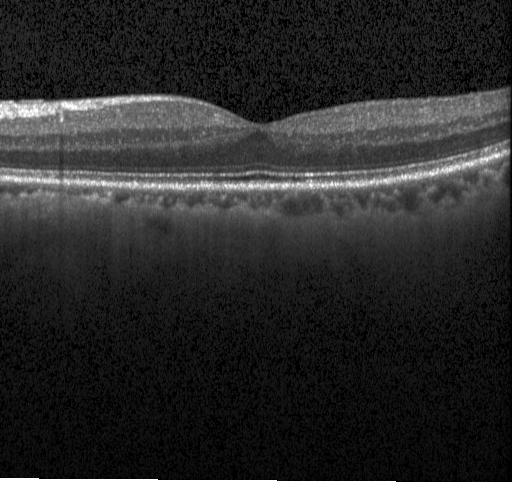 OCT line scan. Spectral-domain optical coherence tomography. Centered on the fovea. Heidelberg Spectralis — Diagnosis: neither choroidal neovascularization, diabetic macular edema, nor drusen.